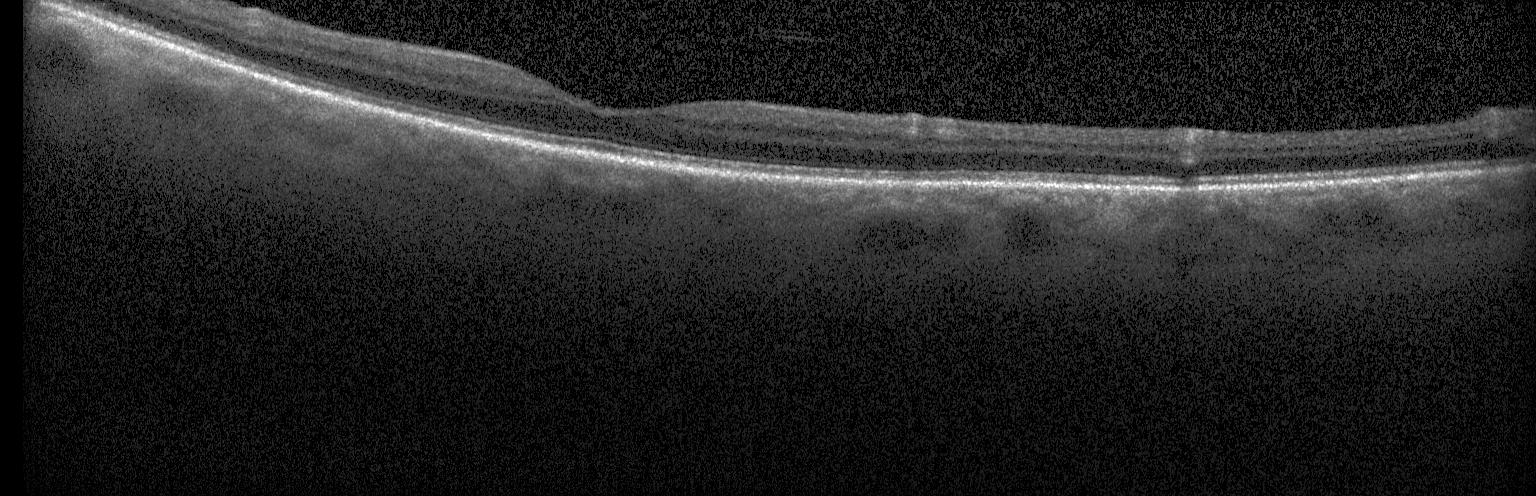
Instrument: Heidelberg Spectralis, retinal OCT cross-section — Dx: no choroidal neovascularization, diabetic macular edema, or drusen.